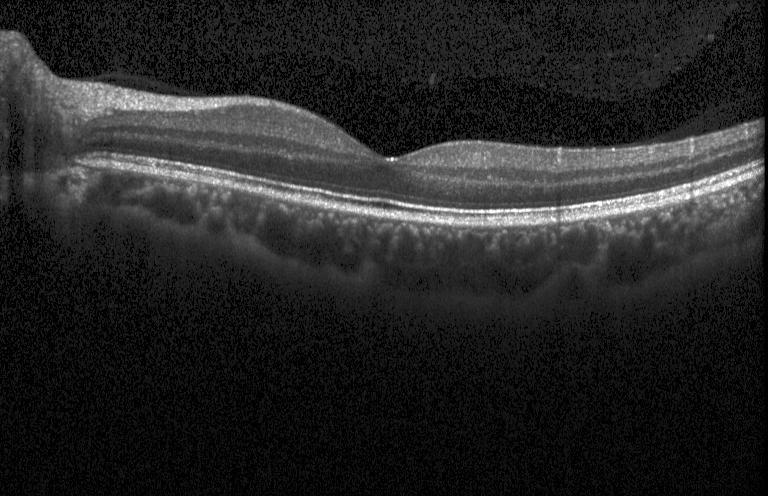 Diagnosis: neither choroidal neovascularization, diabetic macular edema, nor drusen.